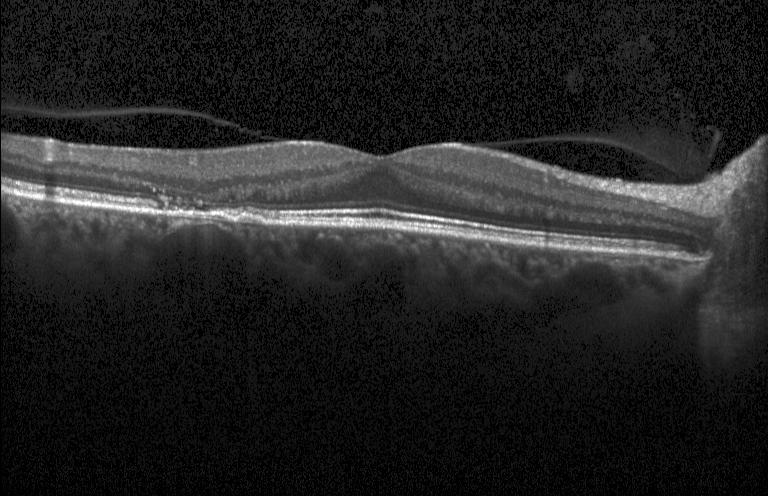
Finding: choroidal neovascularization (CNV).